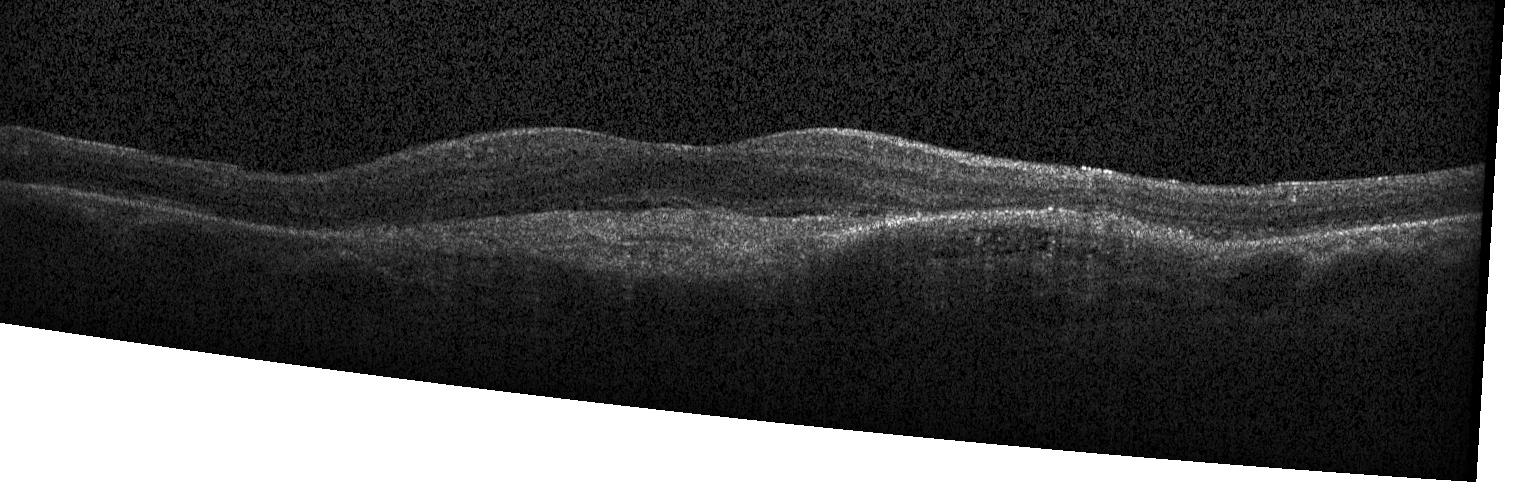 Impression: choroidal neovascularization (CNV).